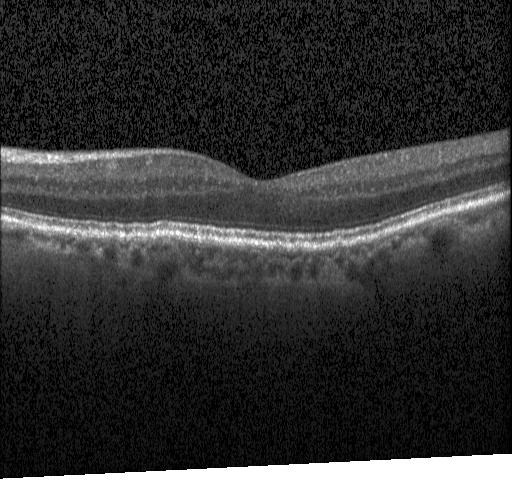

Diagnosis: no CNV, no DME, and no drusen.